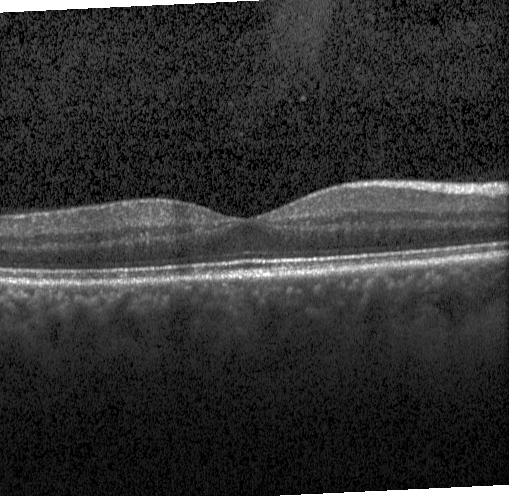

Fovea-centered. OCT line scan. Instrument: Heidelberg Spectralis. Spectral-domain optical coherence tomography
Impression: neither CNV, DME, nor drusen.